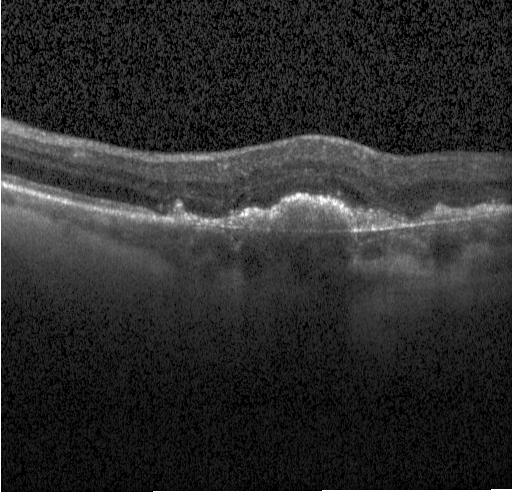 Retinal OCT B-scan; spectral-domain OCT — Finding: a choroidal neovascular membrane.